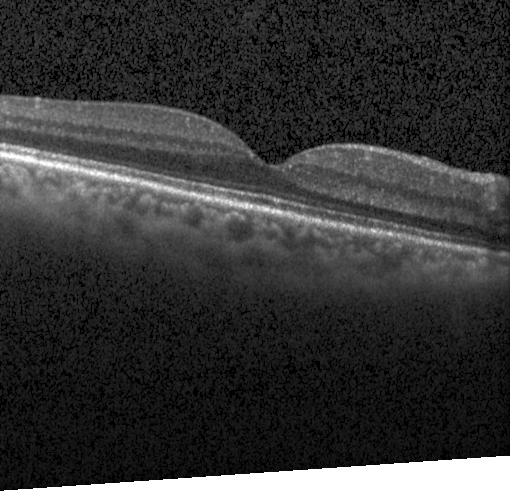 SD-OCT; OCT line scan; macular scan
Macular OCT: no CNV, no DME, and no drusen.